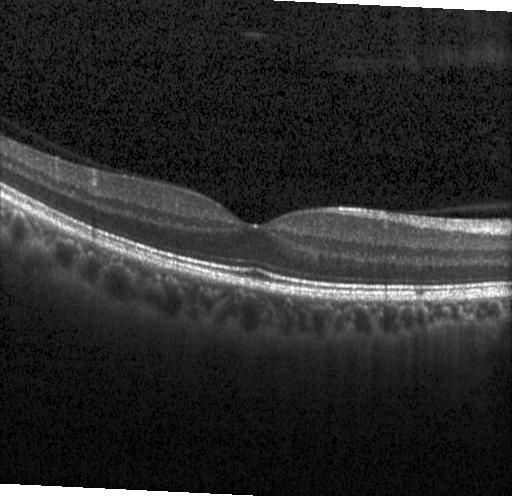
Acquired on a Heidelberg Spectralis · through the macula · spectral-domain OCT · optical coherence tomography scan. The scan shows no choroidal neovascularization, no diabetic macular edema, and no drusen.